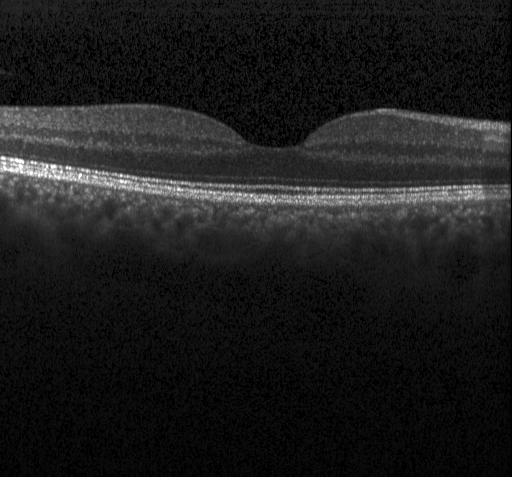

Spectral-domain optical coherence tomography. Heidelberg Spectralis. OCT line scan. Macular scan
Assessment: no CNV, DME, or drusen.